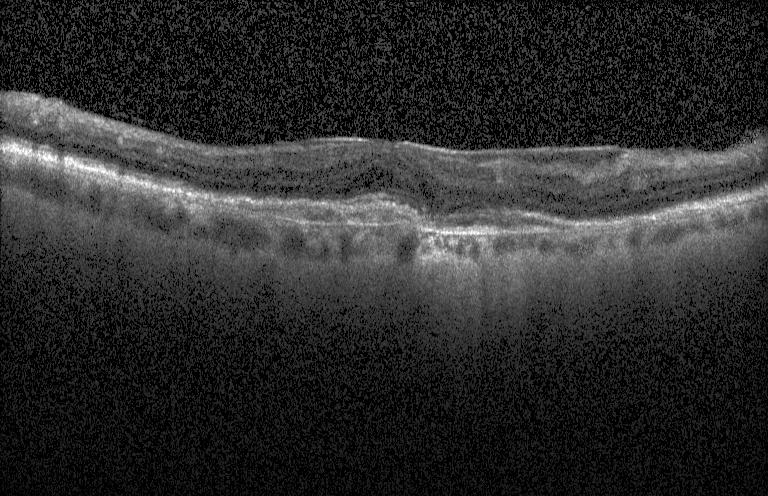 Retinal OCT B-scan — Impression: choroidal neovascularization (CNV).